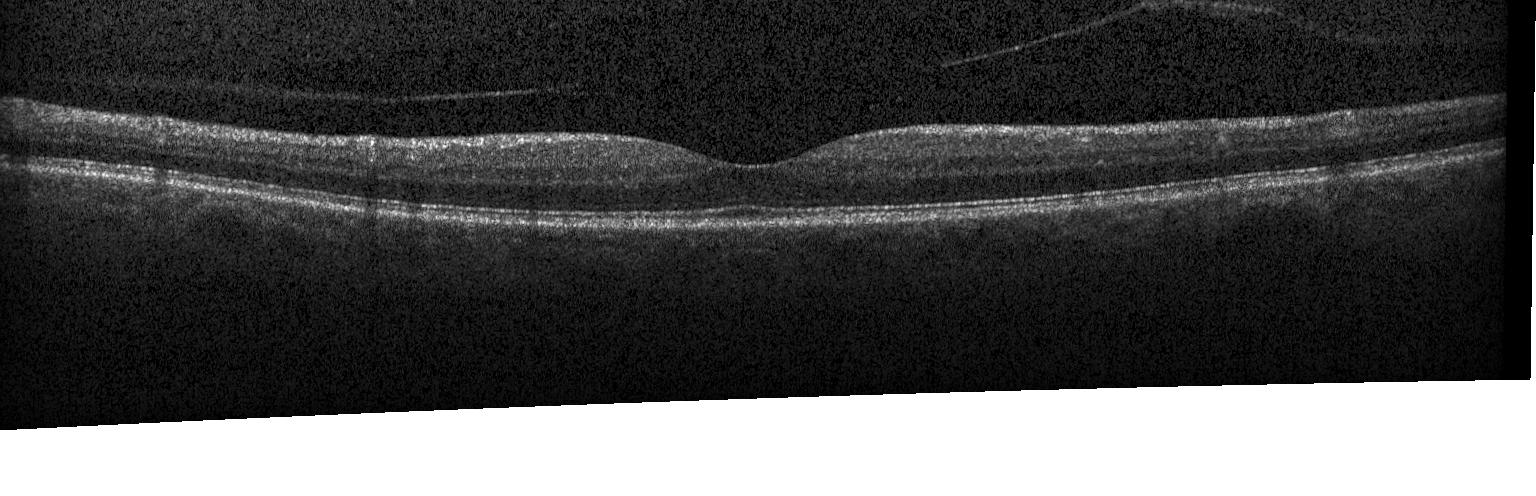
OCT line scan · spectral-domain OCT
This B-scan demonstrates no evidence of CNV, DME, or drusen.